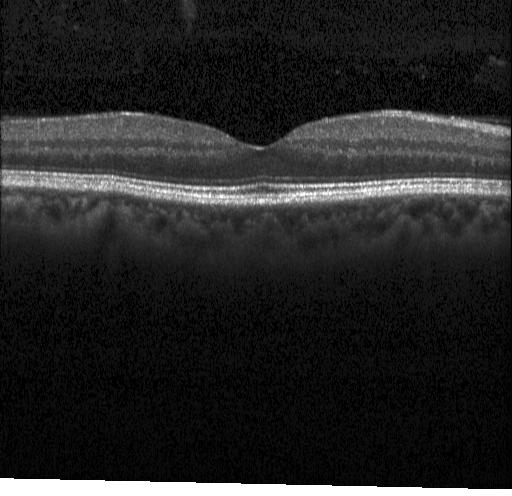
Fovea-centered; SD-OCT; optical coherence tomography B-scan; instrument: Heidelberg Spectralis.
Impression: no choroidal neovascularization, diabetic macular edema, or drusen.